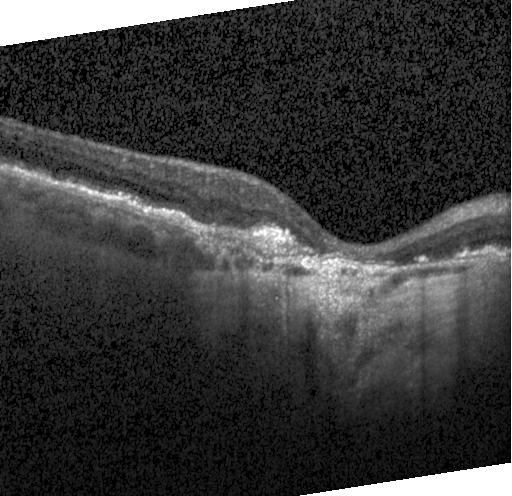 Macular OCT demonstrating a choroidal neovascular membrane.